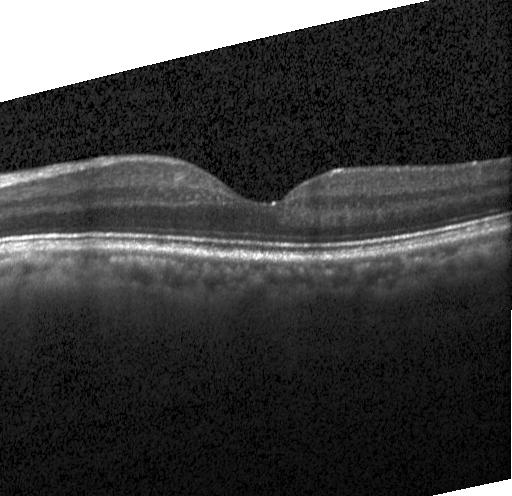
SD-OCT. Optical coherence tomography B-scan. Impression: no choroidal neovascularization, no diabetic macular edema, and no drusen.